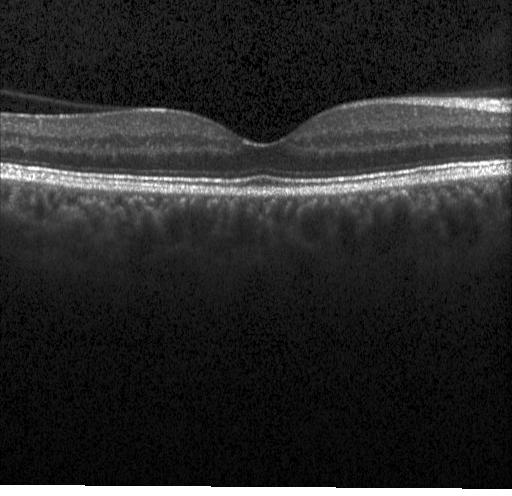

No choroidal neovascularization, no diabetic macular edema, and no drusen.